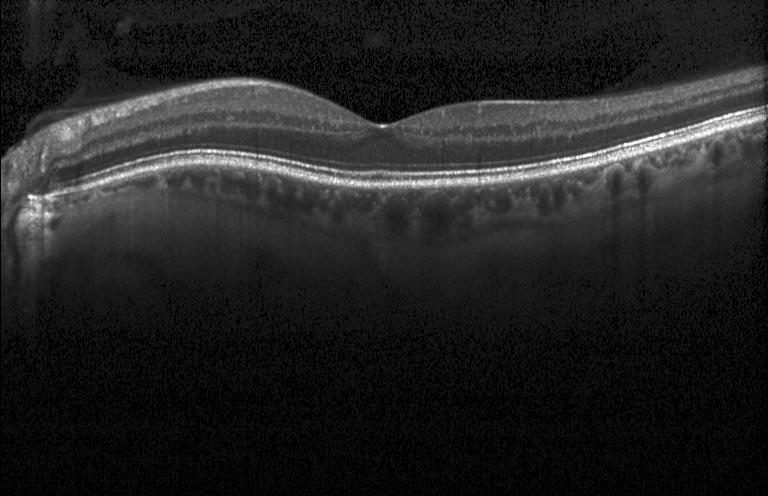

Macular OCT demonstrating no evidence of choroidal neovascularization, diabetic macular edema, or drusen.